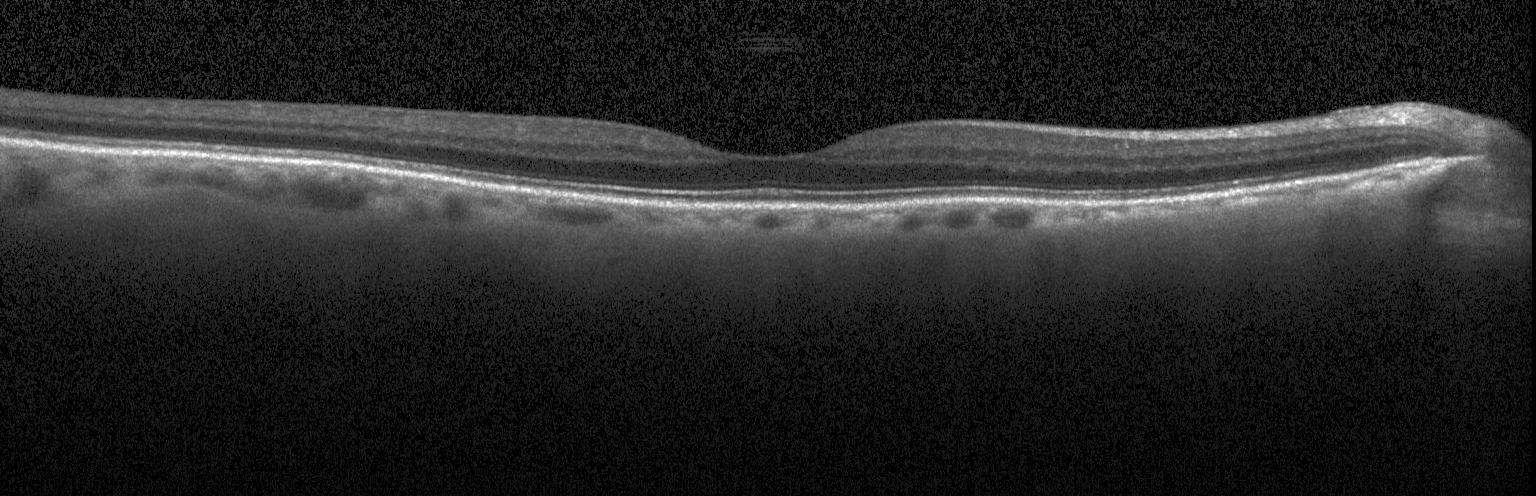

Spectral-domain OCT. Instrument: Heidelberg Spectralis. Retinal OCT B-scan. Finding: no evidence of choroidal neovascularization, diabetic macular edema, or drusen.